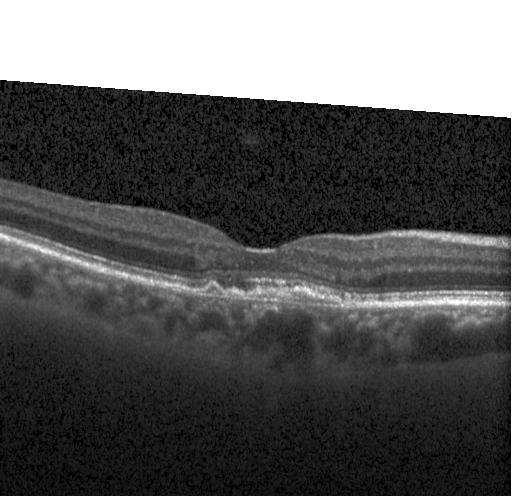
Optical coherence tomography B-scan · spectral-domain optical coherence tomography.
Impression: choroidal neovascularization.